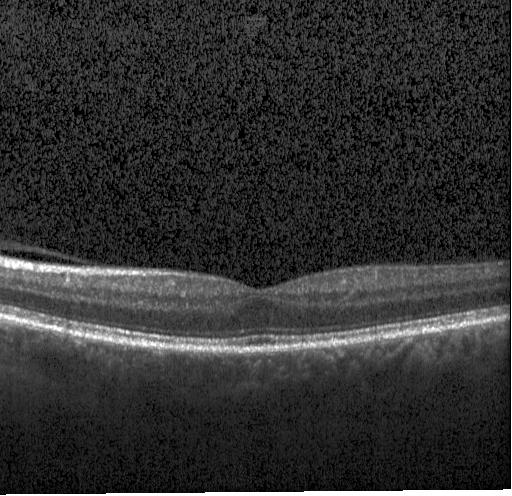

No choroidal neovascularization, no diabetic macular edema, and no drusen.